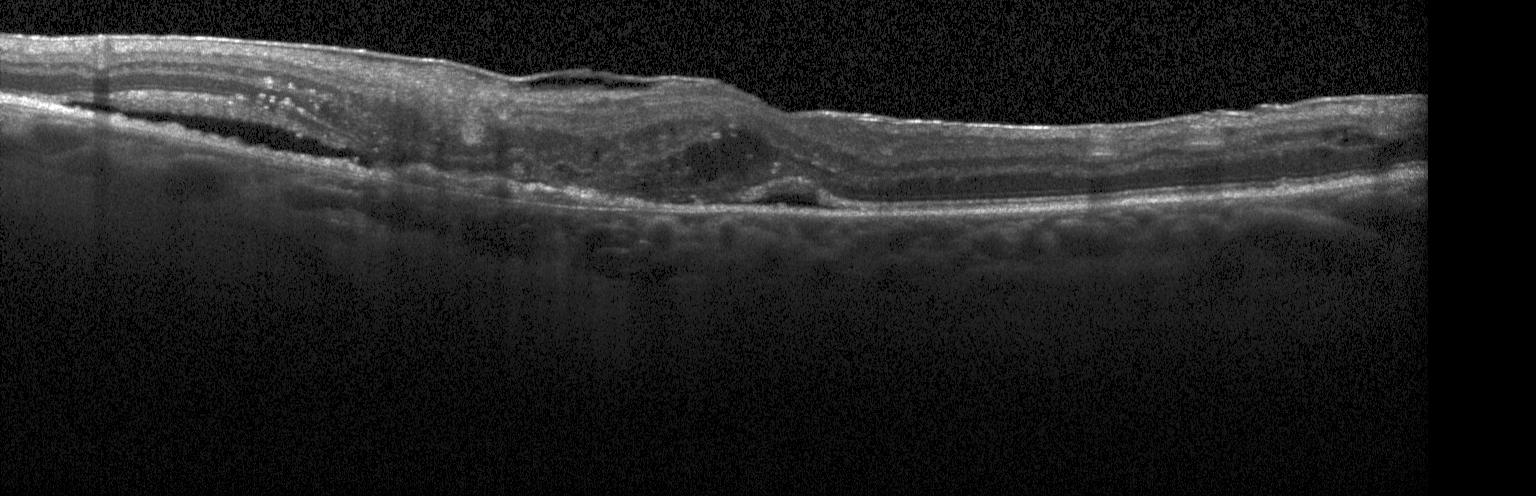
A choroidal neovascular membrane.